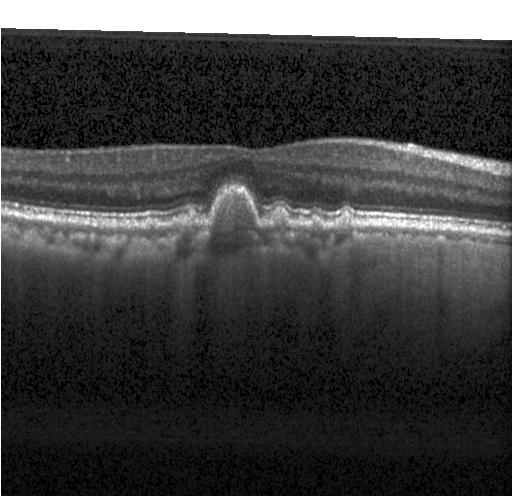

Retinal OCT cross-section showing a choroidal neovascular membrane.